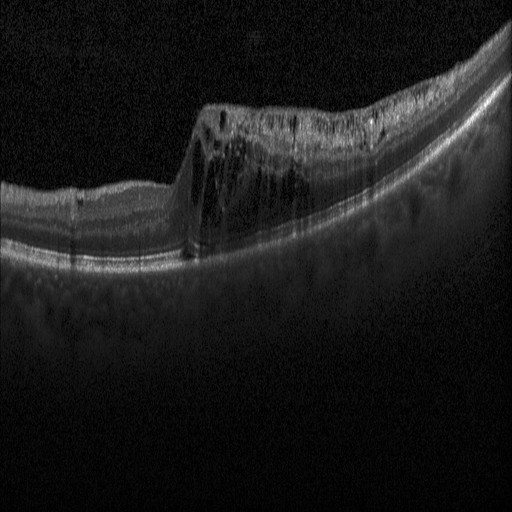
Optical coherence tomography scan — DME.